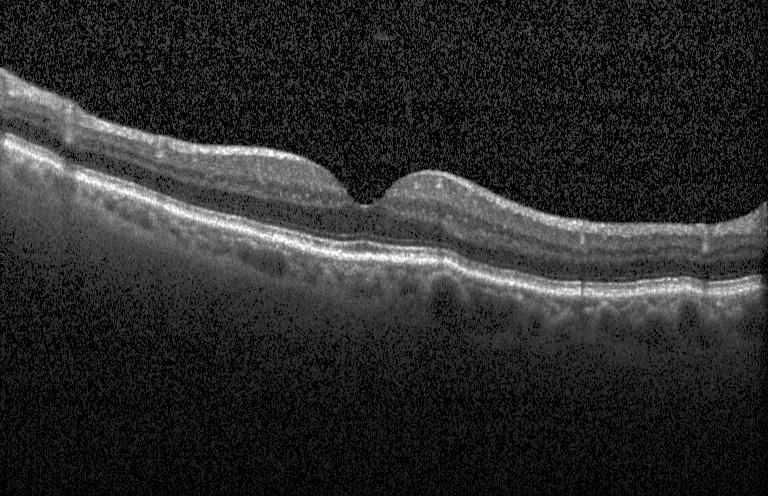
Heidelberg Spectralis. OCT line scan.
Assessment: no CNV, no DME, and no drusen.